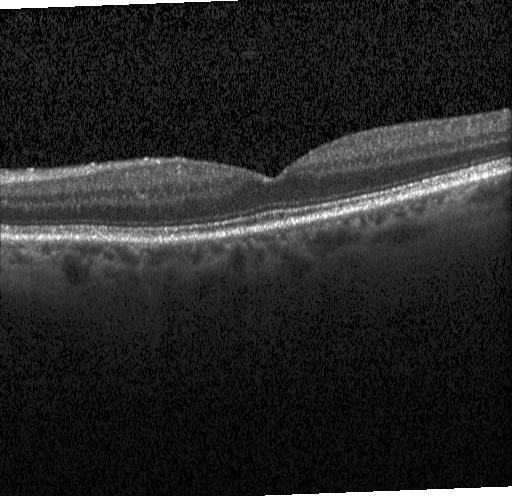
Centered on the fovea, OCT B-scan, Heidelberg Spectralis OCT system. This B-scan demonstrates no evidence of CNV, DME, or drusen.